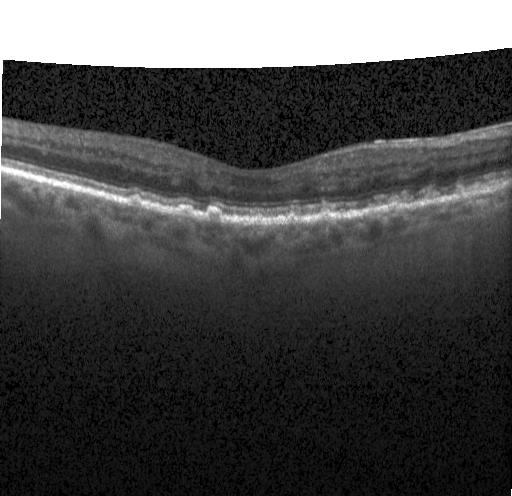 Instrument: Heidelberg Spectralis, retinal OCT B-scan, SD-OCT.
Diagnosis: drusen.